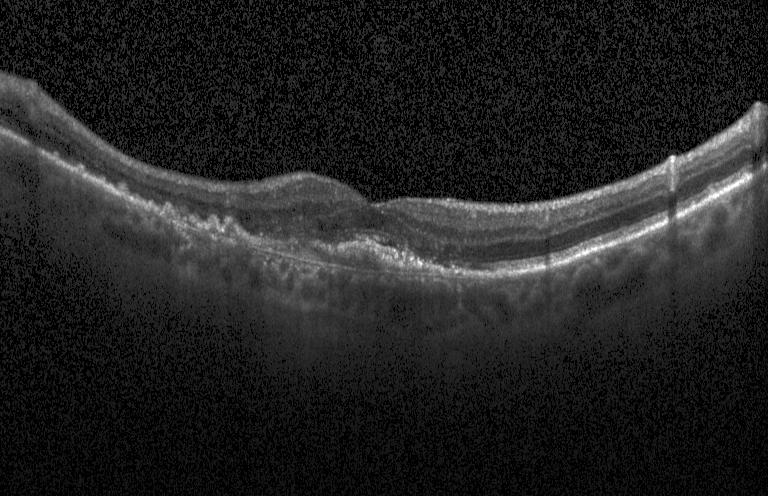
Diagnosis: a choroidal neovascular membrane.